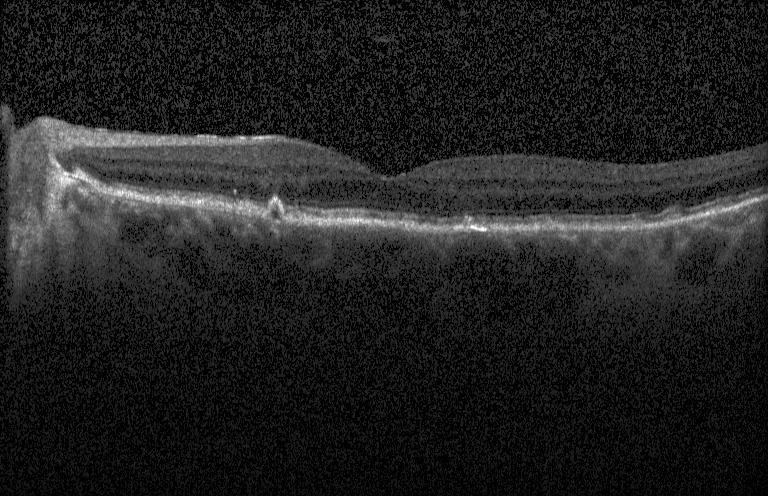

Finding: multiple drusen.